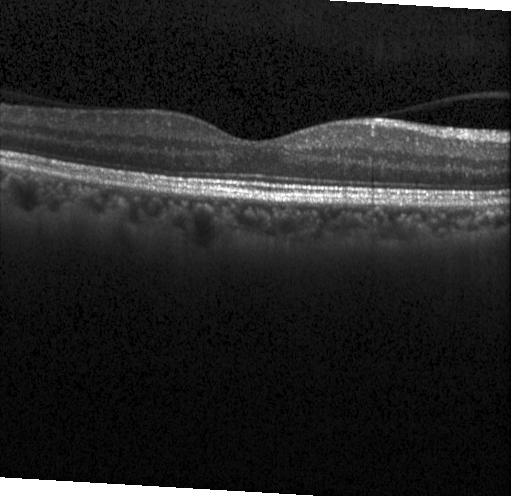

Optical coherence tomography B-scan. OCT finding: no choroidal neovascularization, no diabetic macular edema, and no drusen.